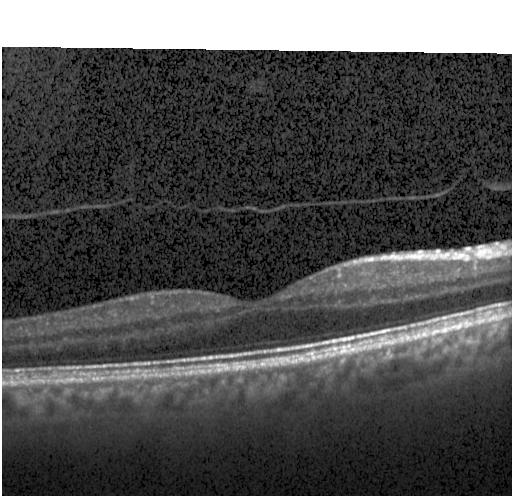 Optical coherence tomography B-scan, spectral-domain optical coherence tomography, macular scan. Neither CNV, DME, nor drusen.